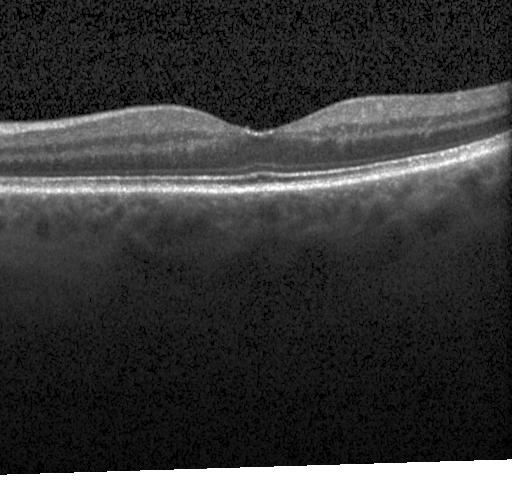

OCT line scan · centered on the fovea · Heidelberg Spectralis OCT system · spectral-domain OCT. Finding: no evidence of choroidal neovascularization, diabetic macular edema, or drusen.